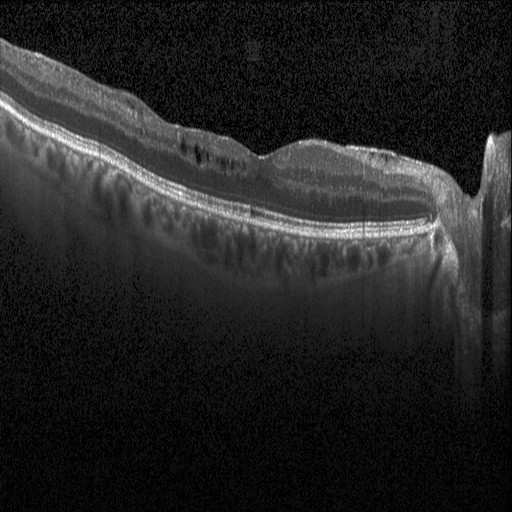
Optical coherence tomography scan, Heidelberg Spectralis OCT system.
OCT finding: diabetic macular edema (DME).